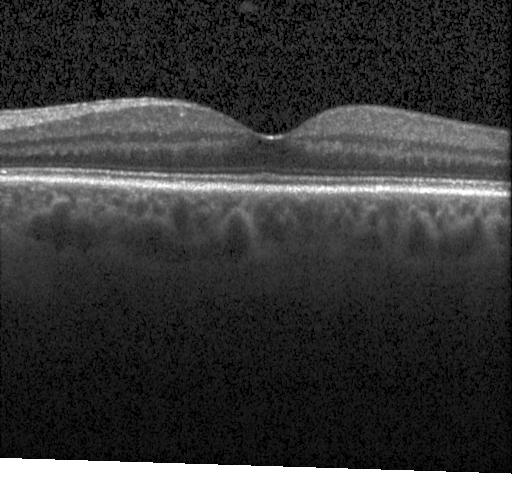
Retinal OCT B-scan; spectral-domain OCT; instrument: Heidelberg Spectralis — Finding: no choroidal neovascularization, no diabetic macular edema, and no drusen.